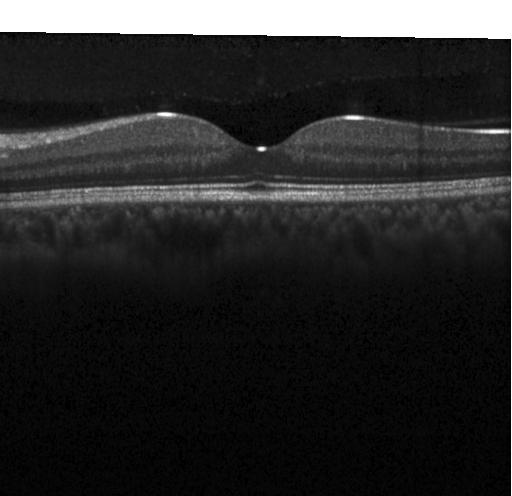

Instrument: Heidelberg Spectralis · OCT B-scan · spectral-domain optical coherence tomography · centered on the fovea. OCT finding: no choroidal neovascularization, diabetic macular edema, or drusen.